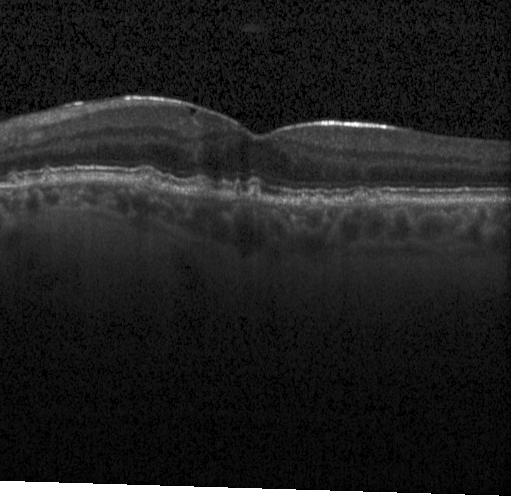 The scan shows sub-RPE drusenoid deposits.